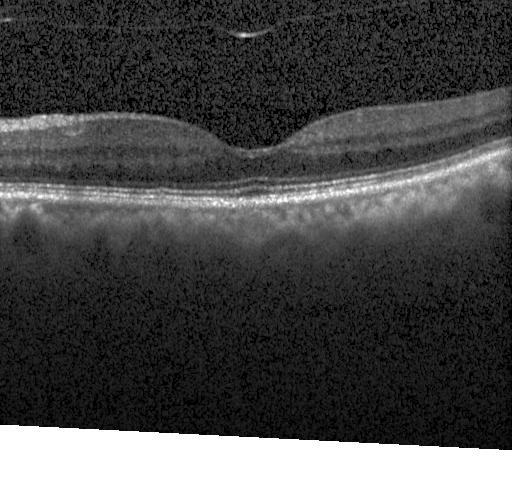 OCT B-scan; through the macula
The scan shows no CNV, DME, or drusen.